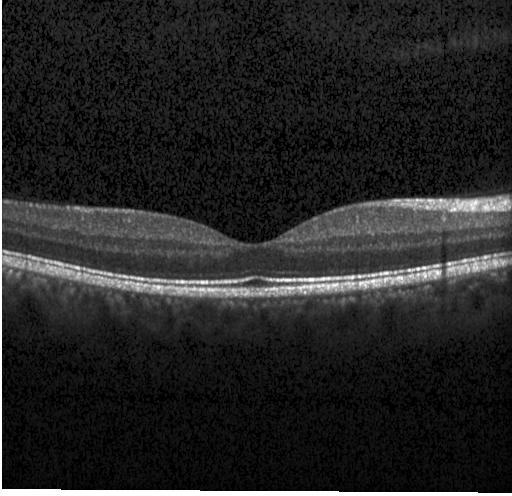

SD-OCT · OCT line scan — Assessment: no choroidal neovascularization, diabetic macular edema, or drusen.